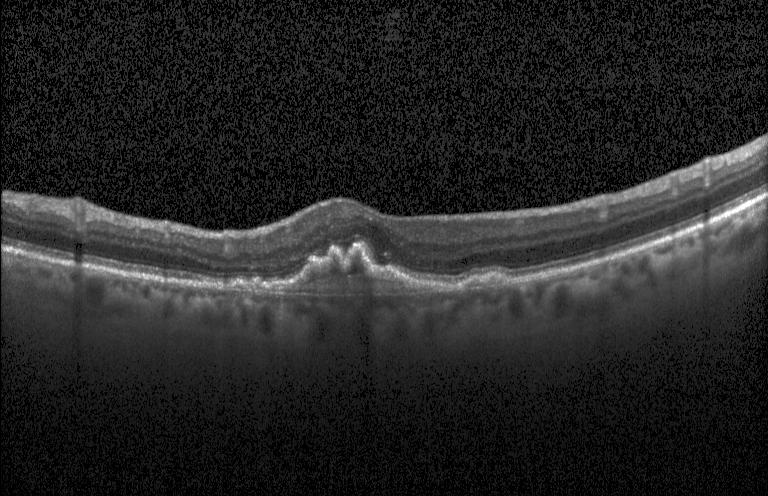

This B-scan demonstrates CNV.